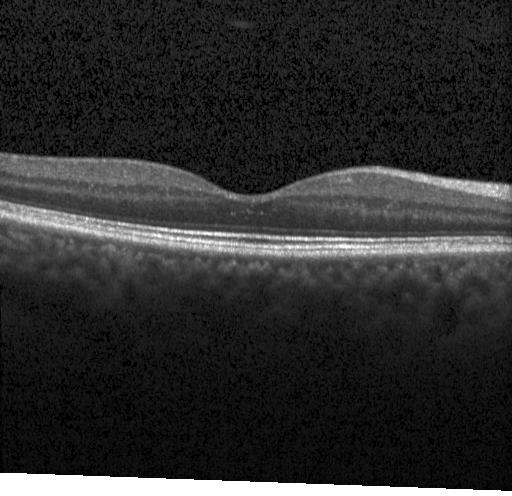

This B-scan demonstrates no choroidal neovascularization, no diabetic macular edema, and no drusen.